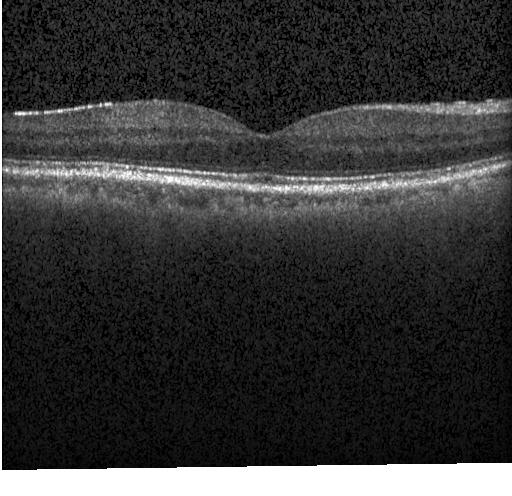 Macular OCT: no CNV, no DME, and no drusen.